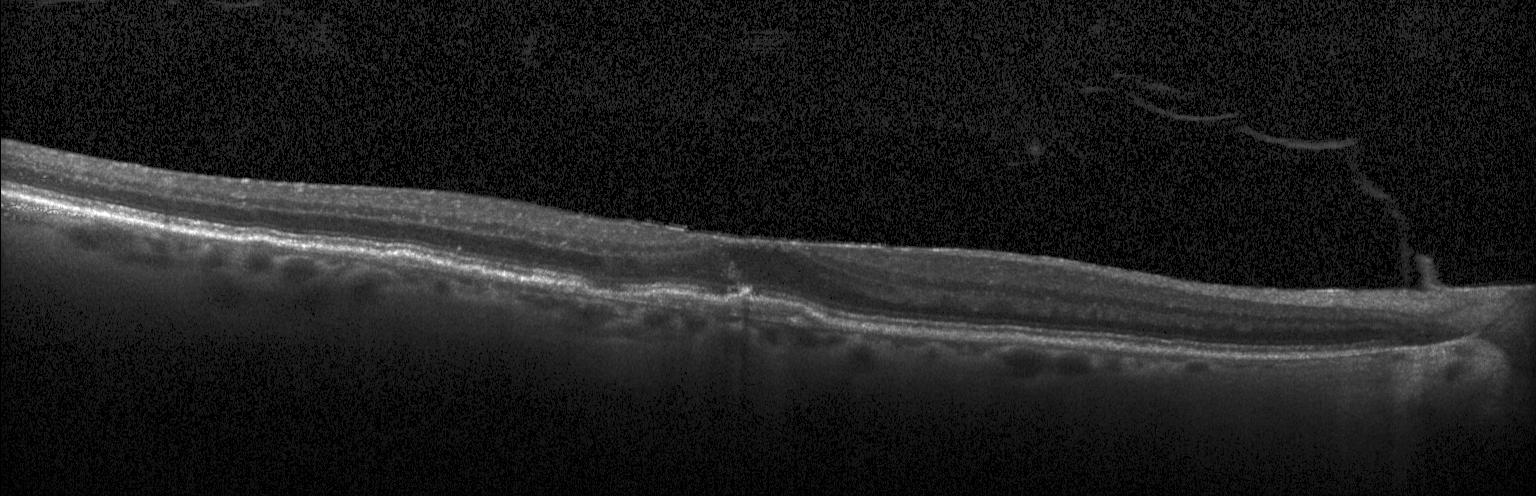
This B-scan demonstrates a choroidal neovascular membrane.